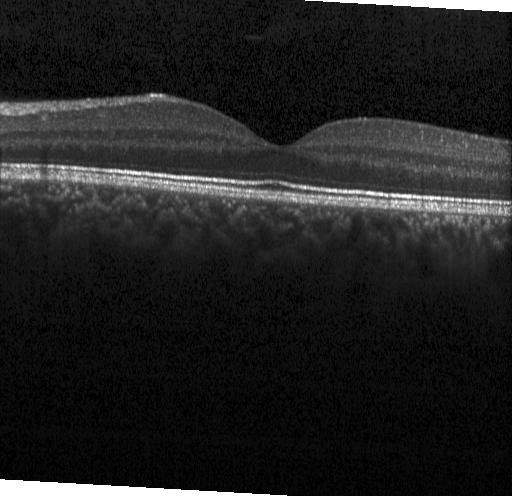

Instrument: Heidelberg Spectralis, fovea-centered, SD-OCT, OCT line scan
Dx: no evidence of choroidal neovascularization, diabetic macular edema, or drusen.